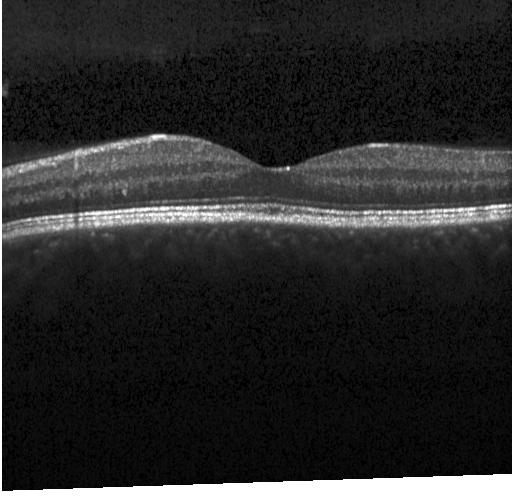

Impression: no evidence of CNV, DME, or drusen.